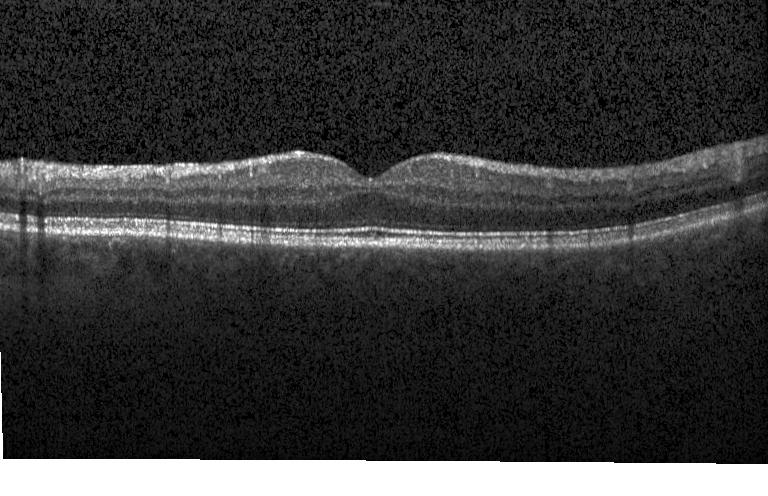
Horizontal scan through the fovea, optical coherence tomography B-scan, spectral-domain optical coherence tomography — Impression: no choroidal neovascularization, diabetic macular edema, or drusen.